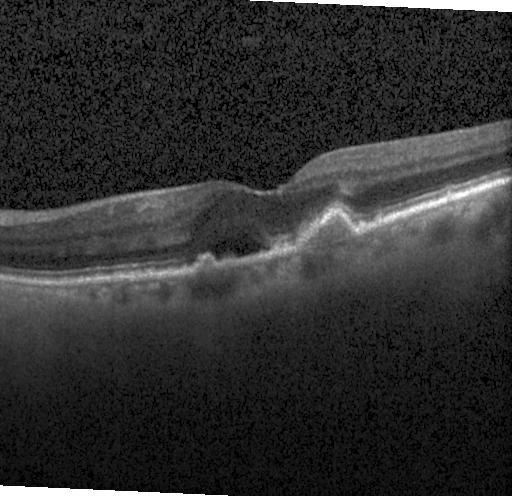 OCT line scan.
Impression: a choroidal neovascular membrane.